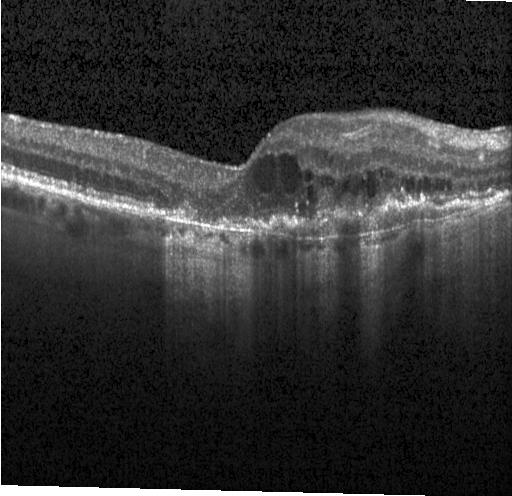

OCT finding: choroidal neovascularization (CNV).